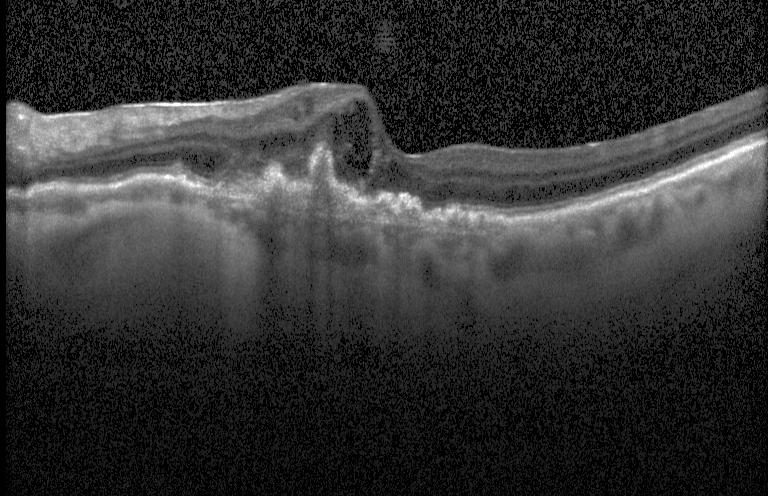

Horizontal scan through the fovea · Heidelberg Spectralis · optical coherence tomography scan · spectral-domain optical coherence tomography — Diagnosis: CNV.